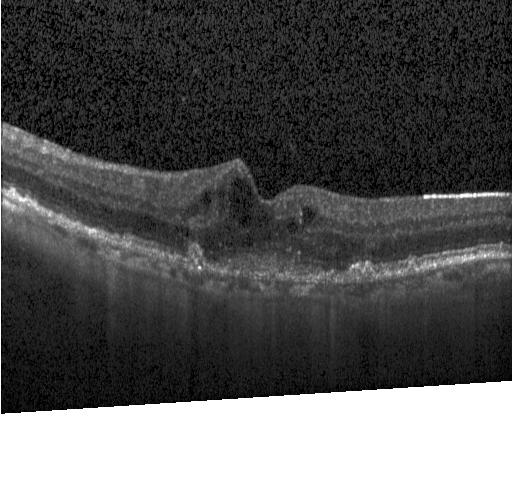
OCT B-scan showing a choroidal neovascular membrane.